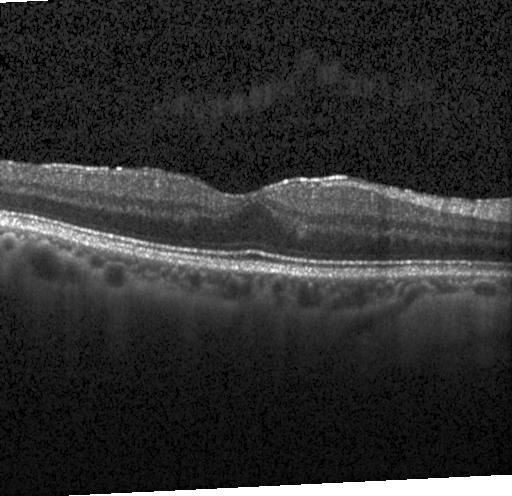

Optical coherence tomography B-scan
Diagnosis: no evidence of choroidal neovascularization, diabetic macular edema, or drusen.